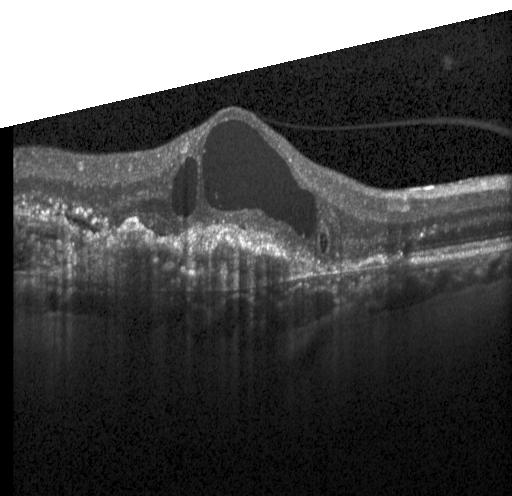 OCT line scan.
Impression: a choroidal neovascular membrane.